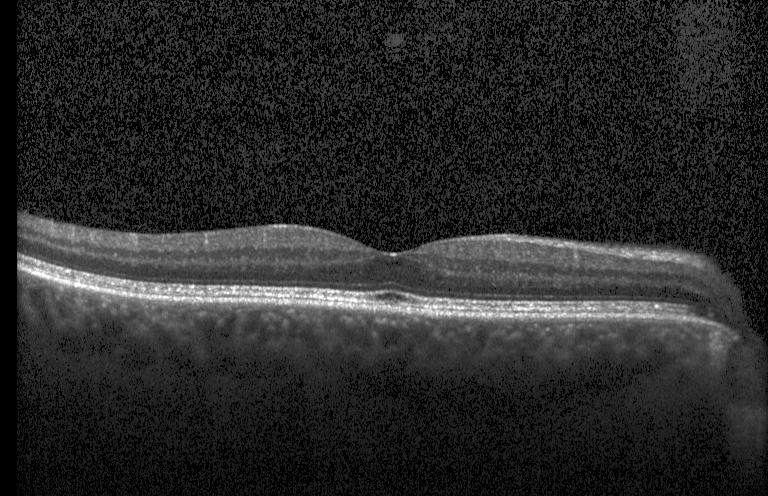 Heidelberg Spectralis OCT system; optical coherence tomography B-scan. Diagnosis: no choroidal neovascularization, diabetic macular edema, or drusen.